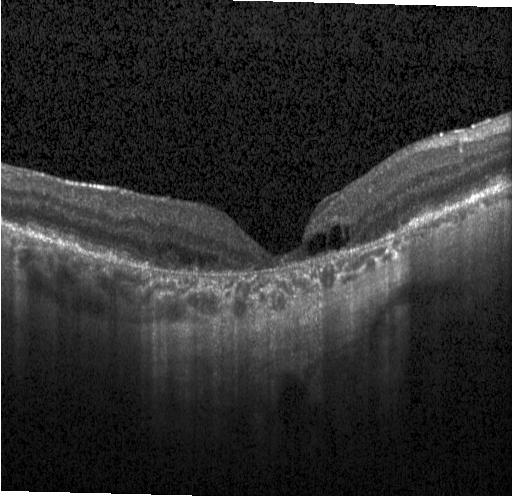
OCT finding: choroidal neovascularization (CNV).